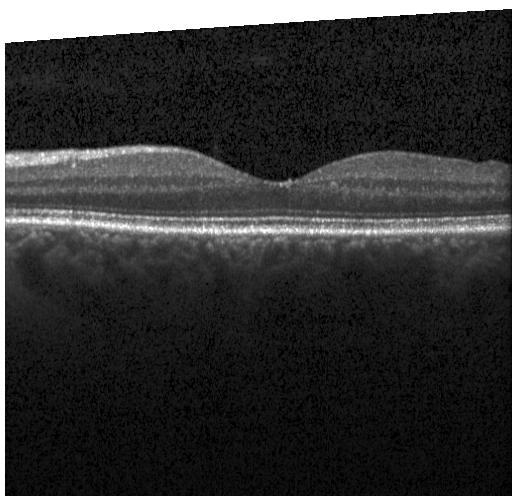
This B-scan demonstrates no evidence of choroidal neovascularization, diabetic macular edema, or drusen.